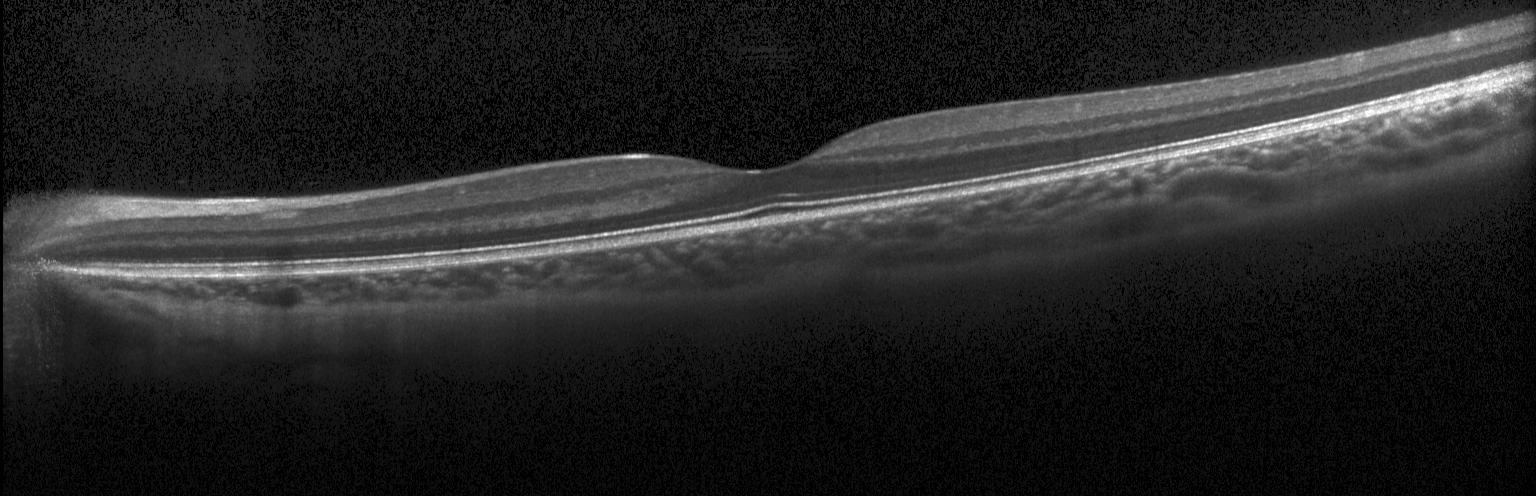
Through the macula · OCT B-scan · spectral-domain OCT · acquired on a Heidelberg Spectralis — Finding: no evidence of choroidal neovascularization, diabetic macular edema, or drusen.